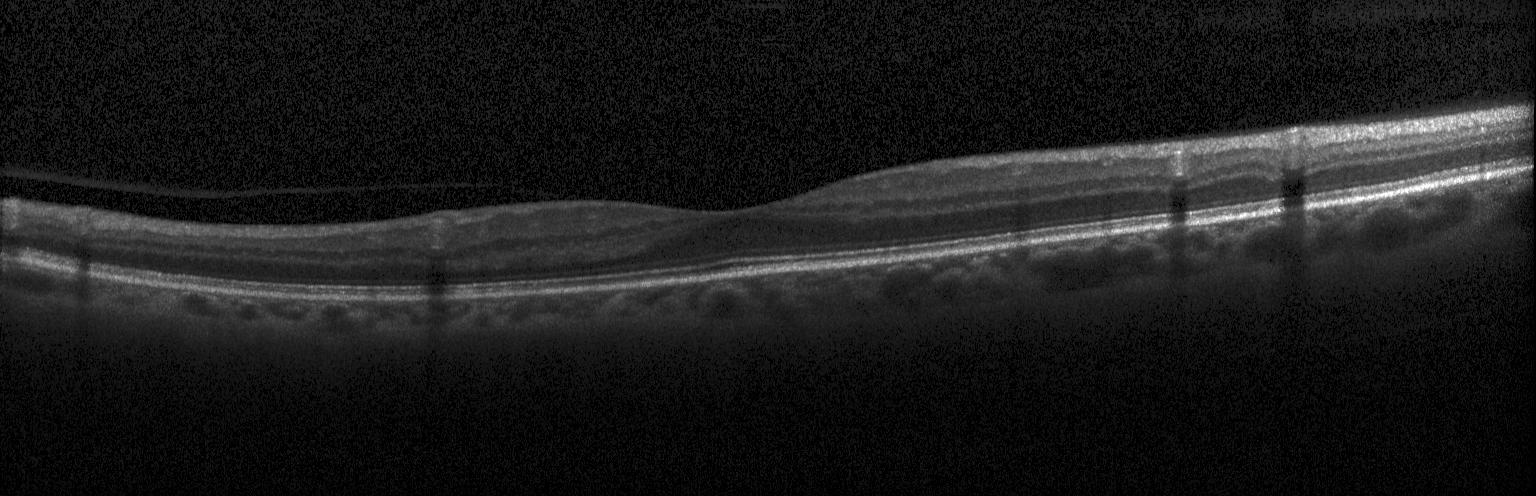 Heidelberg Spectralis OCT system, optical coherence tomography B-scan, spectral-domain optical coherence tomography, through the macula. This B-scan demonstrates neither choroidal neovascularization, diabetic macular edema, nor drusen.